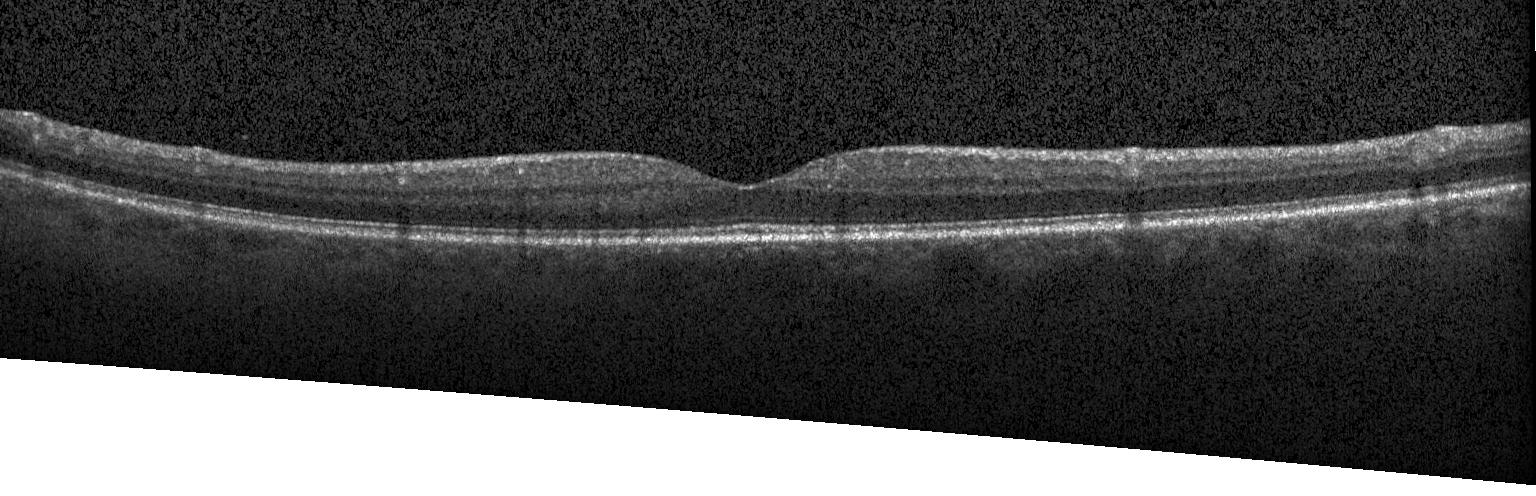 Fovea-centered; Heidelberg Spectralis; spectral-domain optical coherence tomography; optical coherence tomography scan
Neither CNV, DME, nor drusen.